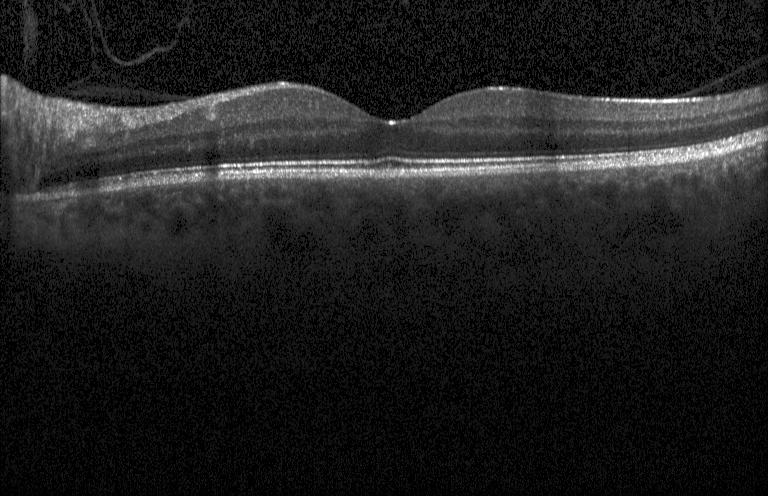 Optical coherence tomography scan, horizontal scan through the fovea, SD-OCT. This B-scan demonstrates no choroidal neovascularization, no diabetic macular edema, and no drusen.